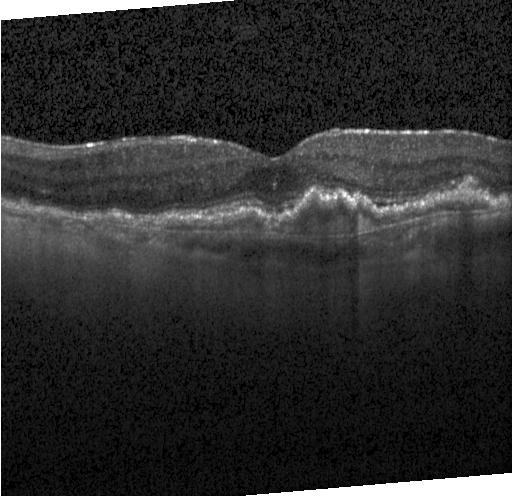

OCT B-scan showing a choroidal neovascular membrane.